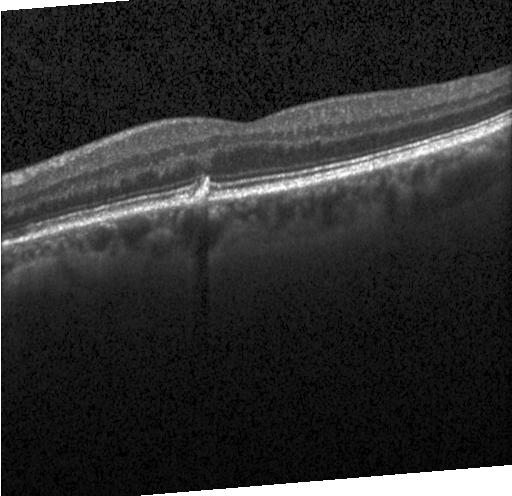
Assessment: CNV.